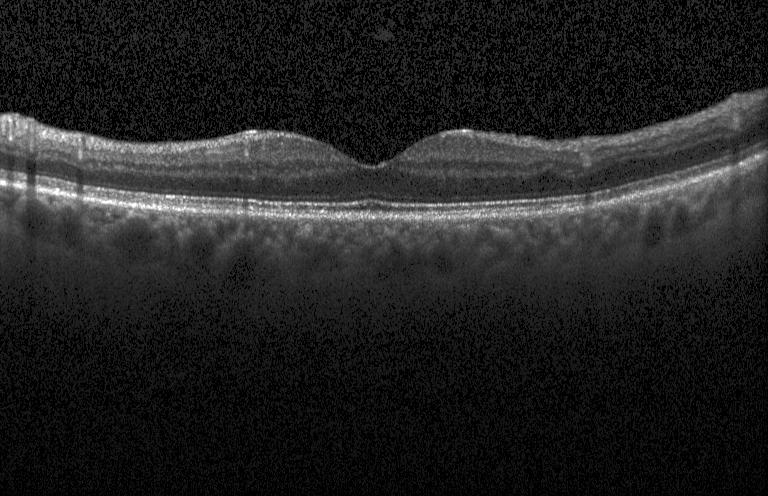 OCT finding: no CNV, DME, or drusen.